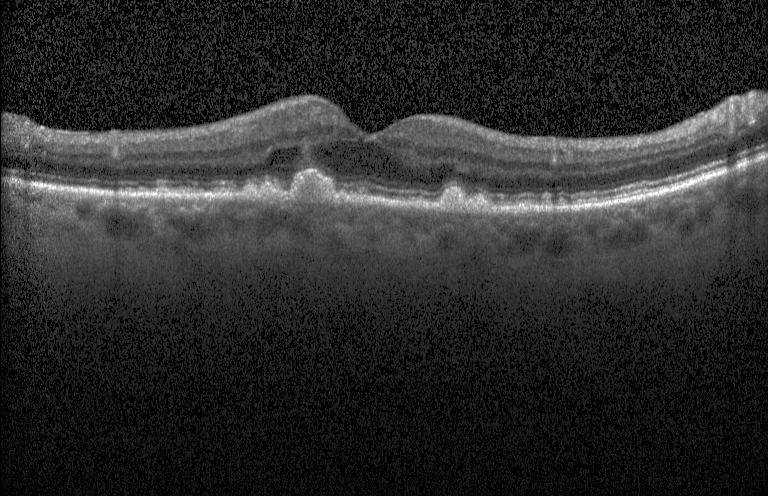
Impression: multiple drusen.